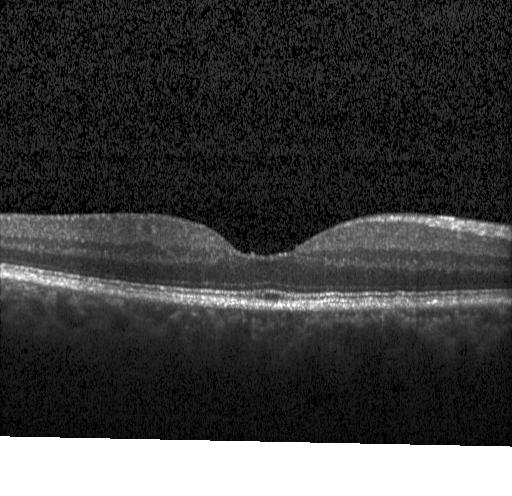 Retinal OCT cross-section; spectral-domain optical coherence tomography; fovea-centered
Diagnosis: no evidence of choroidal neovascularization, diabetic macular edema, or drusen.